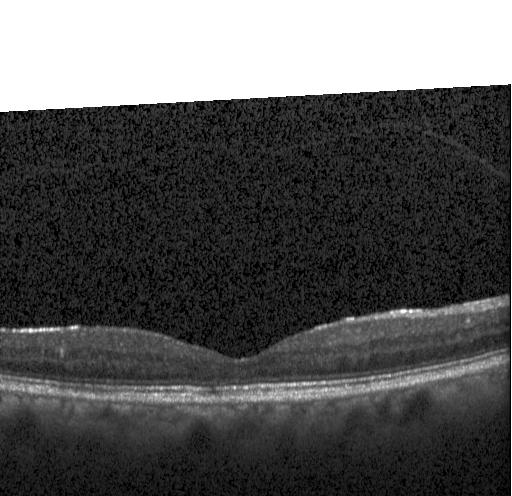

Retinal OCT B-scan. Spectral-domain optical coherence tomography. Through the macula. Instrument: Heidelberg Spectralis.
Assessment: no choroidal neovascularization, no diabetic macular edema, and no drusen.